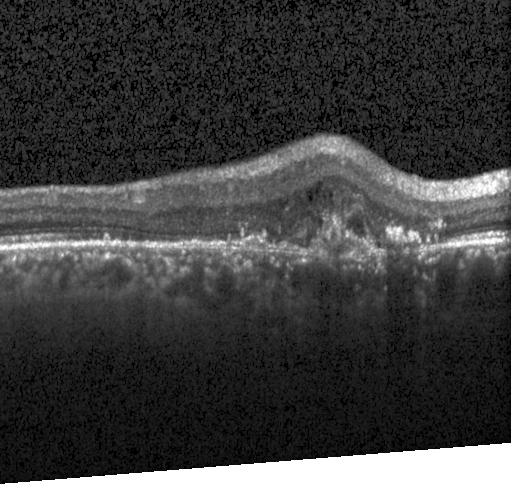 This B-scan demonstrates a choroidal neovascular membrane.